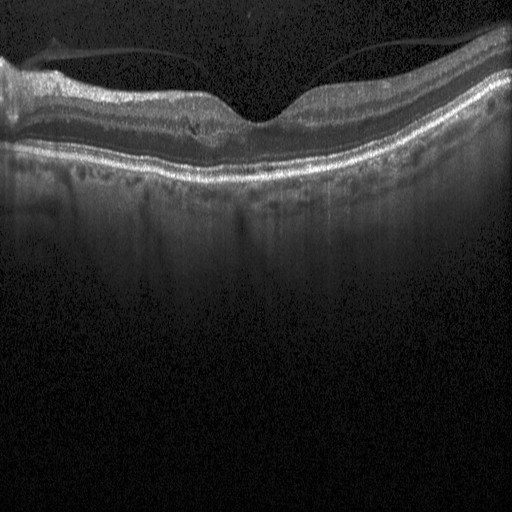
Macular OCT demonstrating DME.